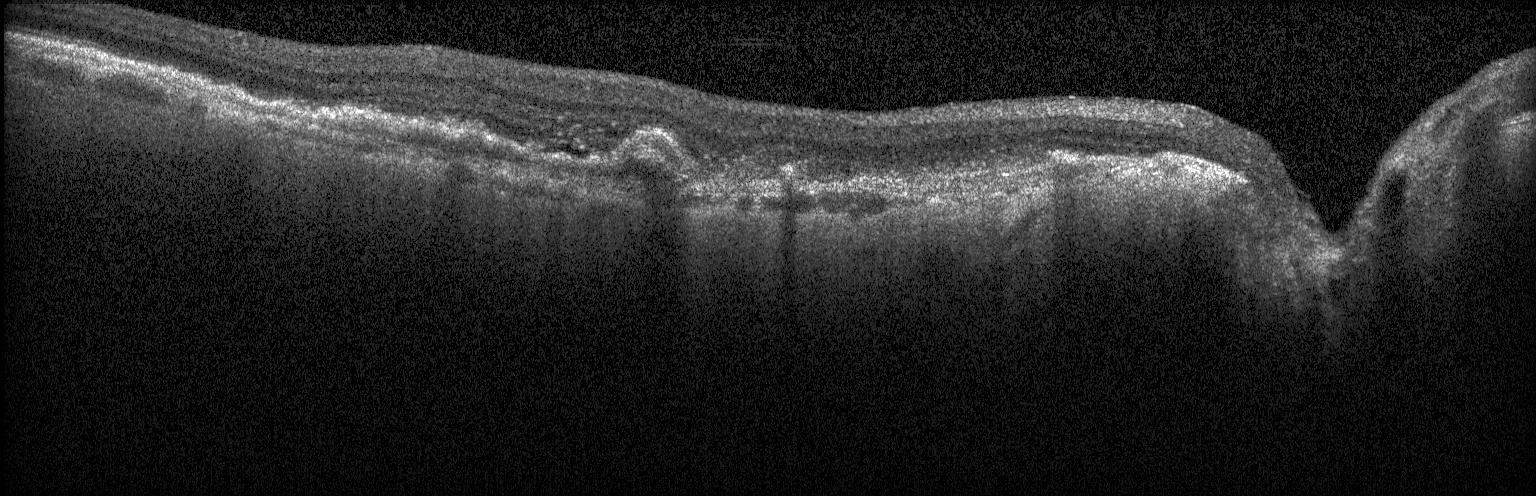

Finding: CNV.